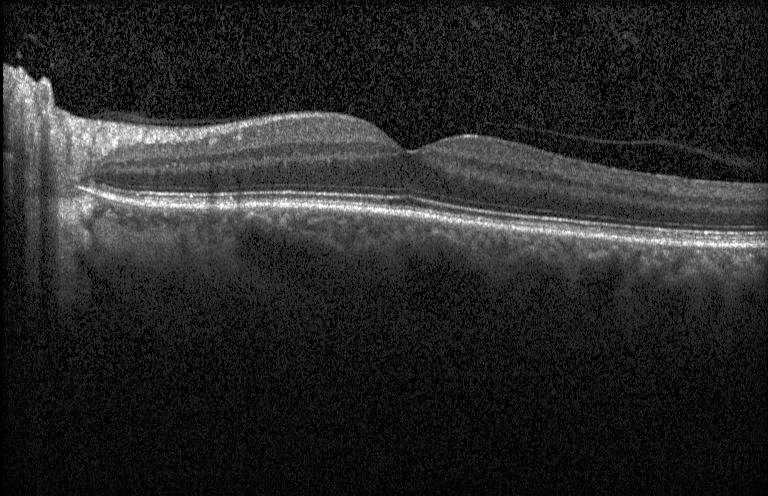
Horizontal scan through the fovea, retinal OCT cross-section, spectral-domain optical coherence tomography.
Diagnosis: no evidence of choroidal neovascularization, diabetic macular edema, or drusen.